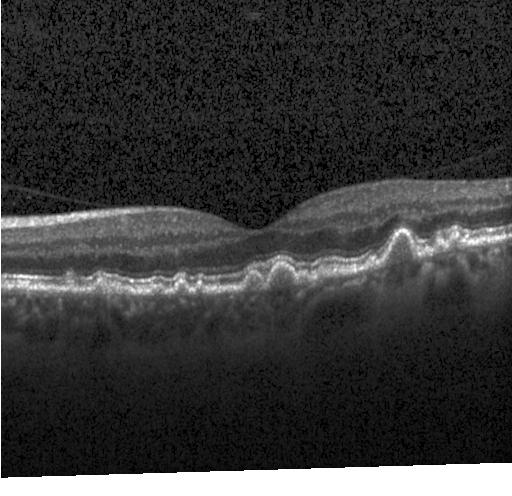
Dx: drusen.